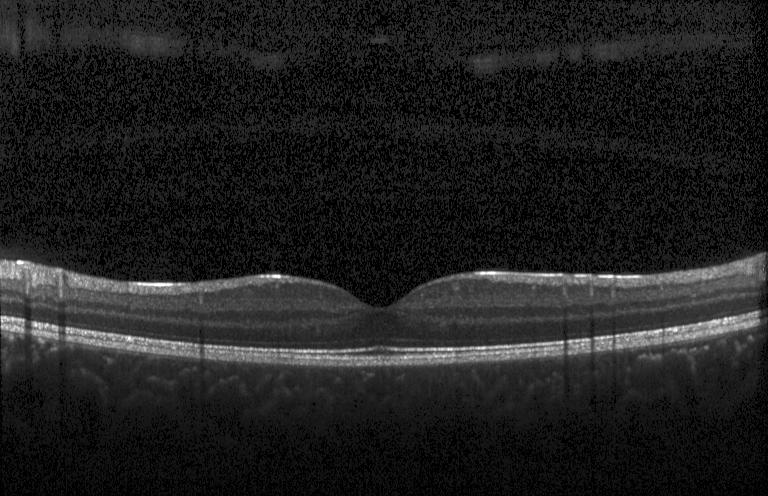

Impression: no choroidal neovascularization, diabetic macular edema, or drusen.